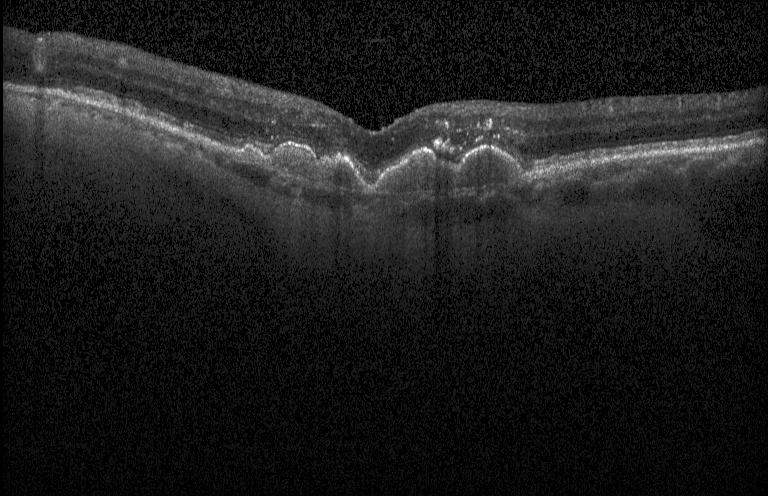 Finding: a choroidal neovascular membrane.